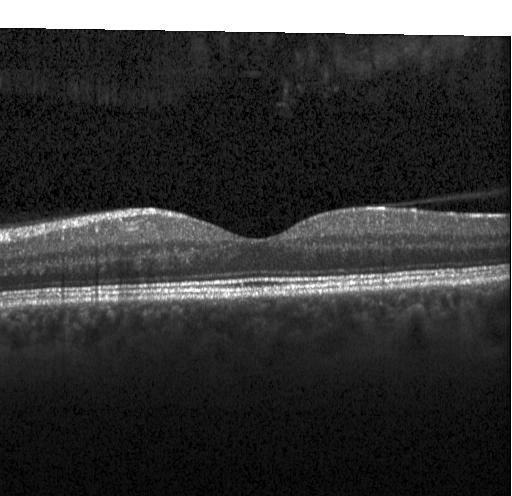
Retinal OCT cross-section. Diagnosis: no choroidal neovascularization, no diabetic macular edema, and no drusen.